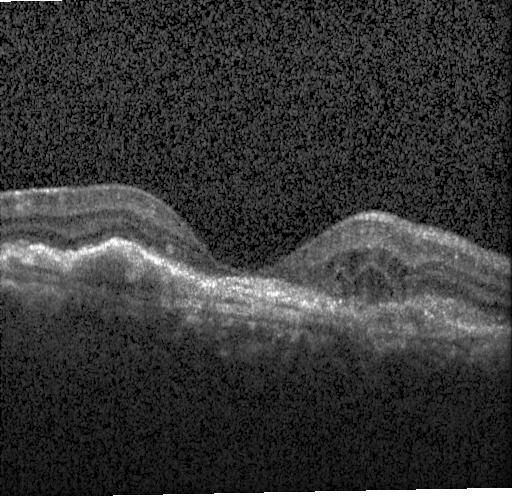

Diagnosis: a choroidal neovascular membrane.